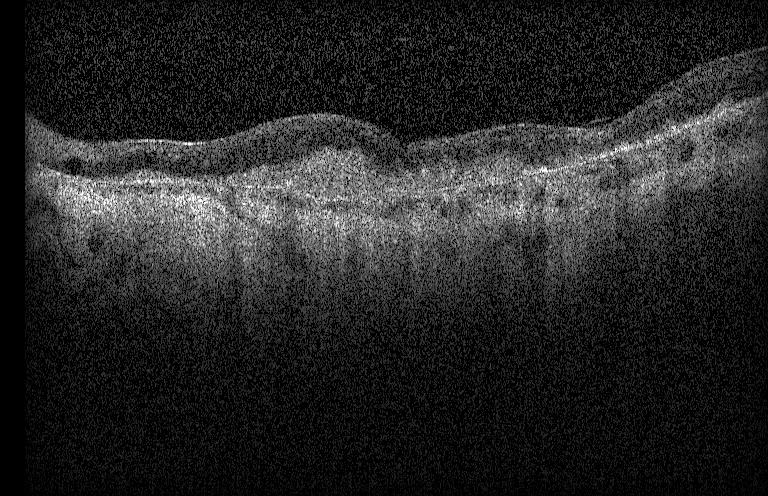

Impression: a choroidal neovascular membrane.